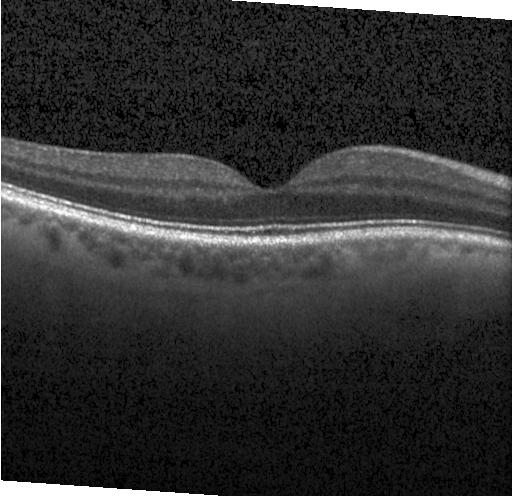

Optical coherence tomography scan
Dx: neither CNV, DME, nor drusen.